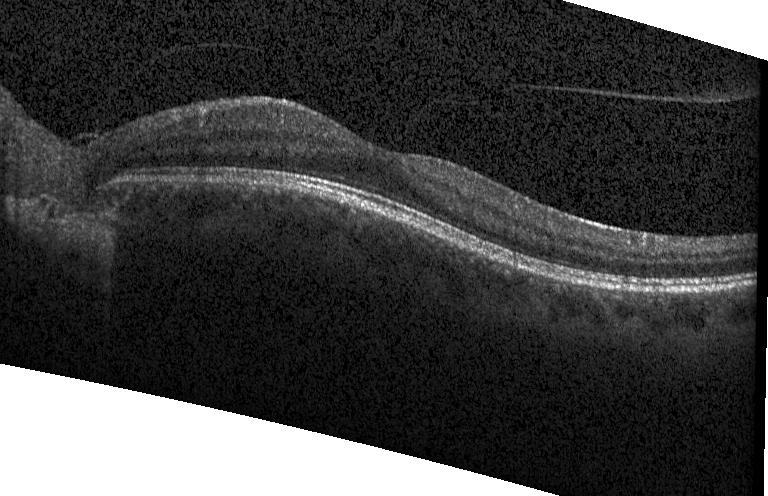
Spectral-domain OCT, optical coherence tomography scan — This B-scan demonstrates no CNV, no DME, and no drusen.